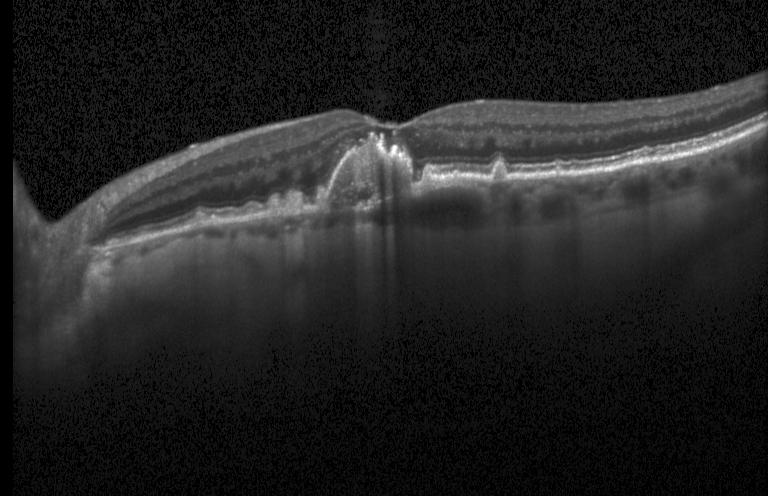
Horizontal scan through the fovea. OCT line scan.
Impression: CNV.